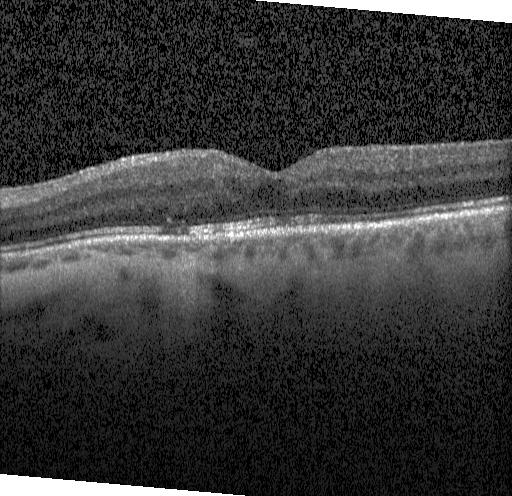 The scan shows no CNV, no DME, and no drusen.